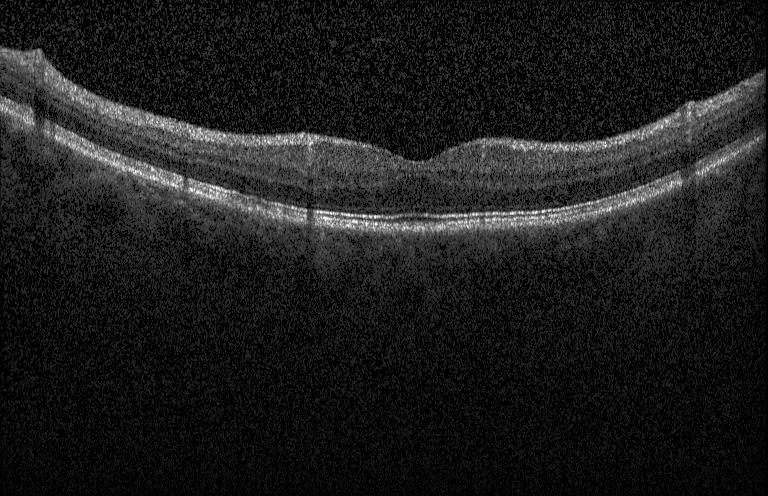

OCT line scan — Diagnosis: no CNV, DME, or drusen.